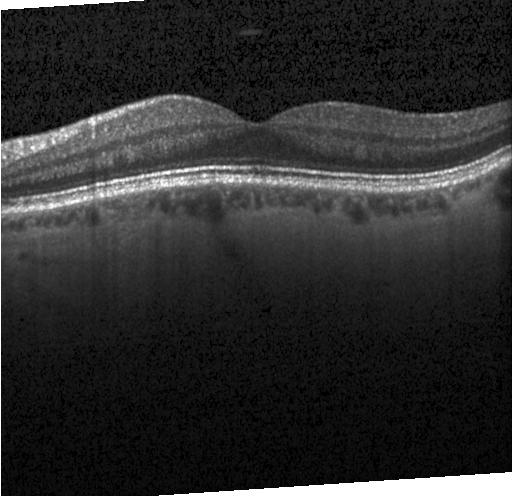
OCT B-scan
The scan shows no evidence of CNV, DME, or drusen.